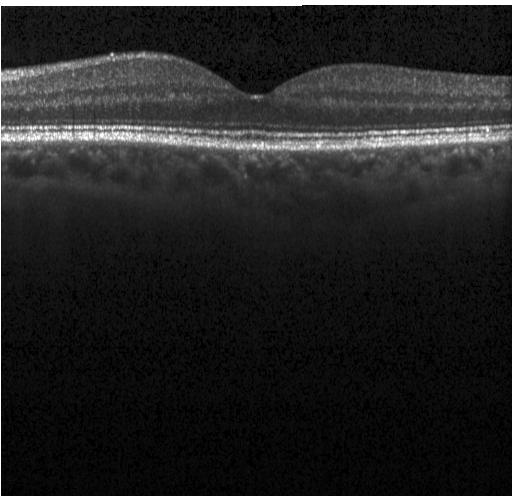

OCT B-scan. Heidelberg Spectralis. Spectral-domain OCT. Finding: no CNV, DME, or drusen.